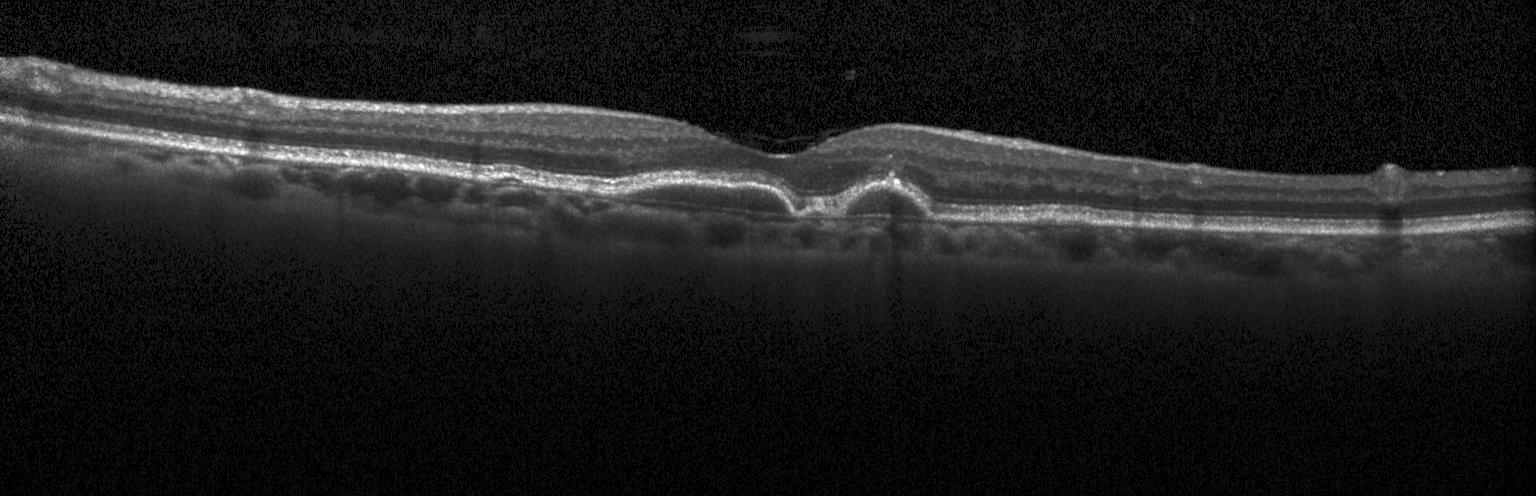
Centered on the fovea, optical coherence tomography scan
This B-scan demonstrates CNV.